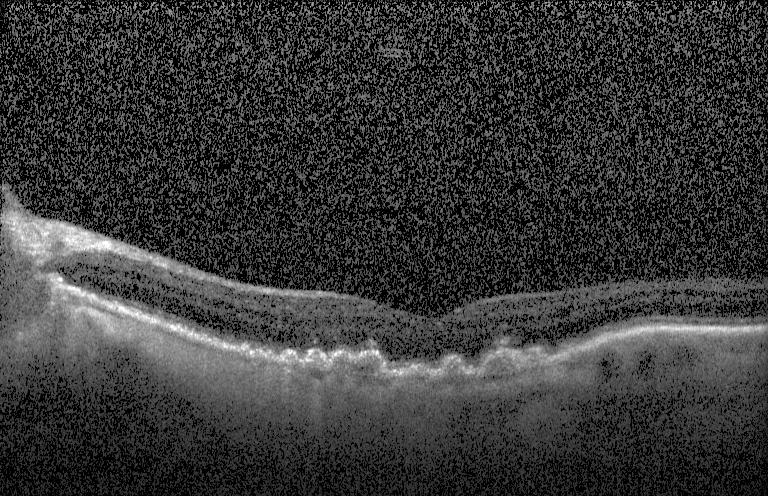 Spectral-domain OCT · optical coherence tomography scan — Finding: sub-RPE drusenoid deposits.